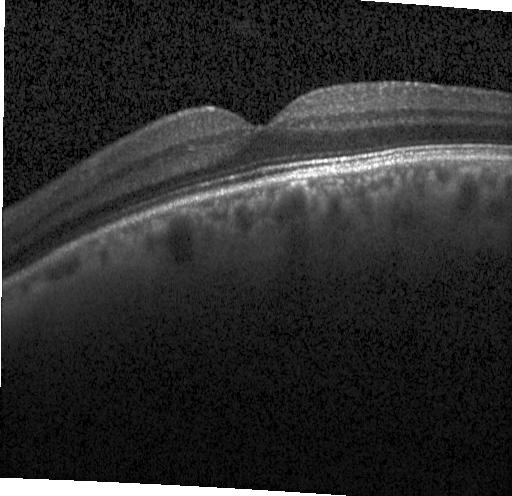

OCT finding: no CNV, no DME, and no drusen.